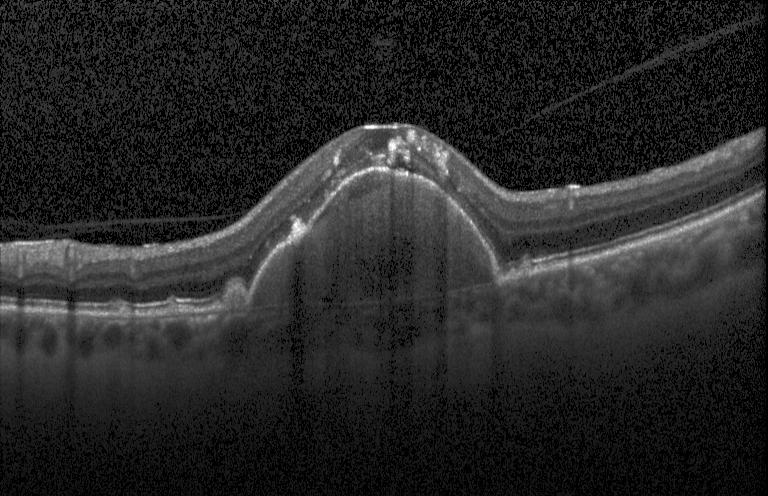
Fovea-centered. SD-OCT. Retinal OCT cross-section. Acquired on a Heidelberg Spectralis.
Diagnosis: a choroidal neovascular membrane.